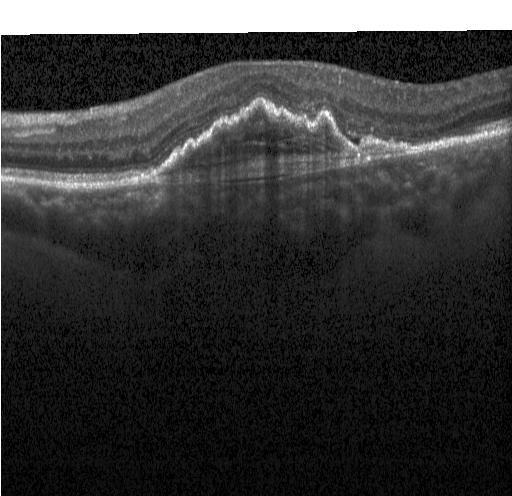
OCT finding: a choroidal neovascular membrane.